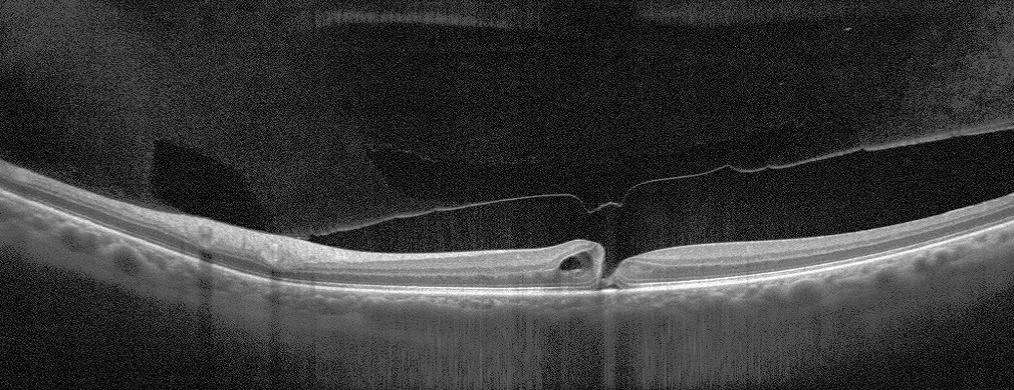

Oculus sinister; retinal OCT B-scan.
Finding: vitreomacular interface disease (VID).